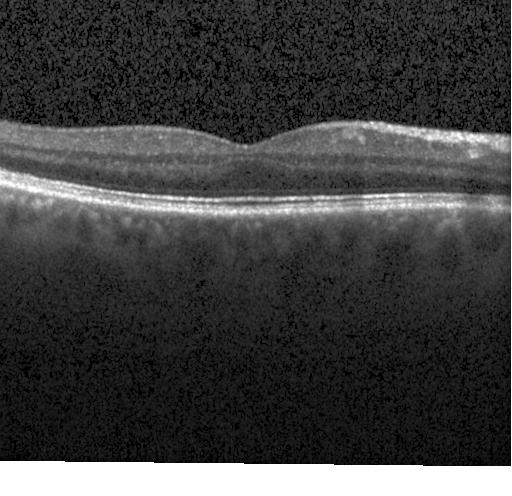
Dx: no evidence of CNV, DME, or drusen.